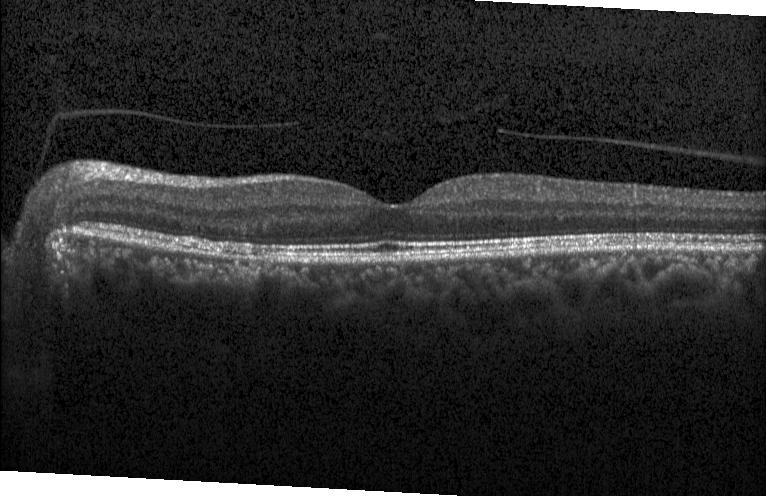 Diagnosis: no evidence of CNV, DME, or drusen.